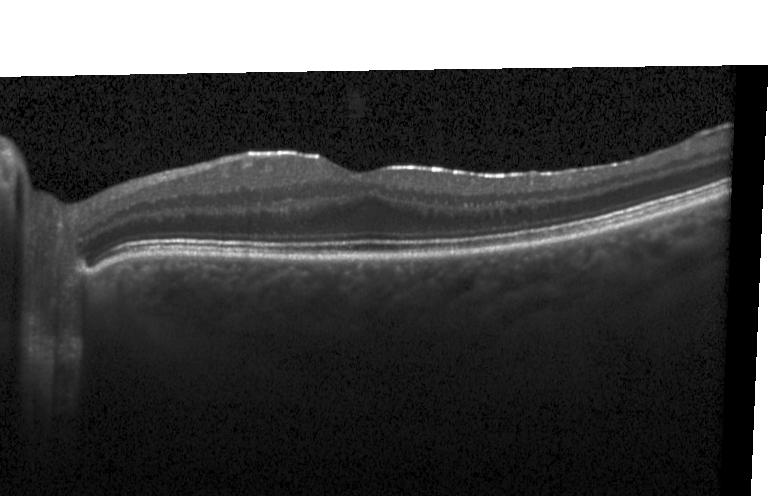
Finding: no choroidal neovascularization, no diabetic macular edema, and no drusen.